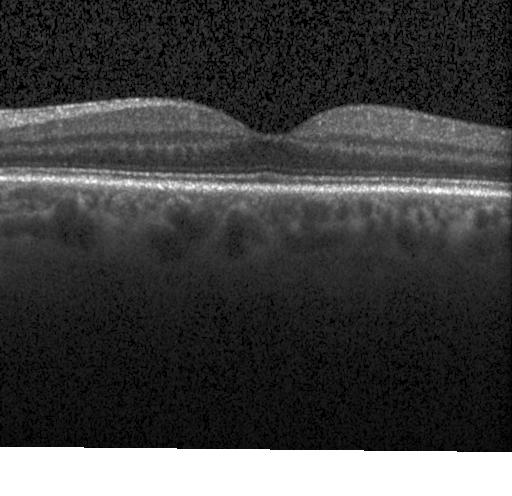
Macular OCT: no evidence of choroidal neovascularization, diabetic macular edema, or drusen.